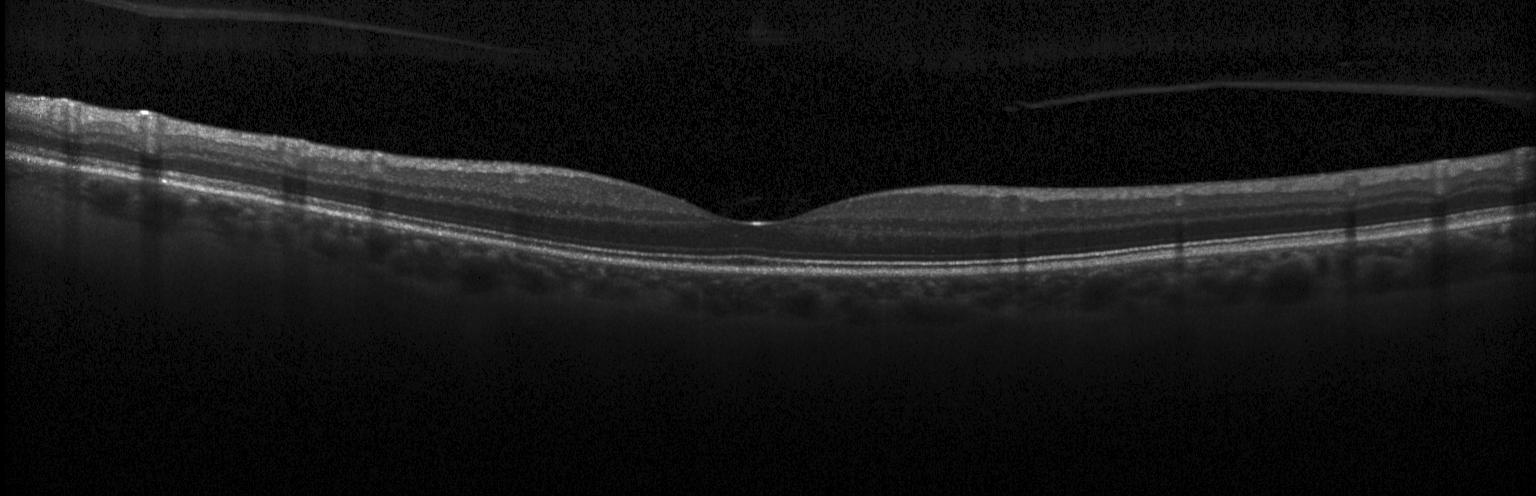 Instrument: Heidelberg Spectralis; SD-OCT; through the macula; retinal OCT cross-section — Macular OCT: no CNV, no DME, and no drusen.